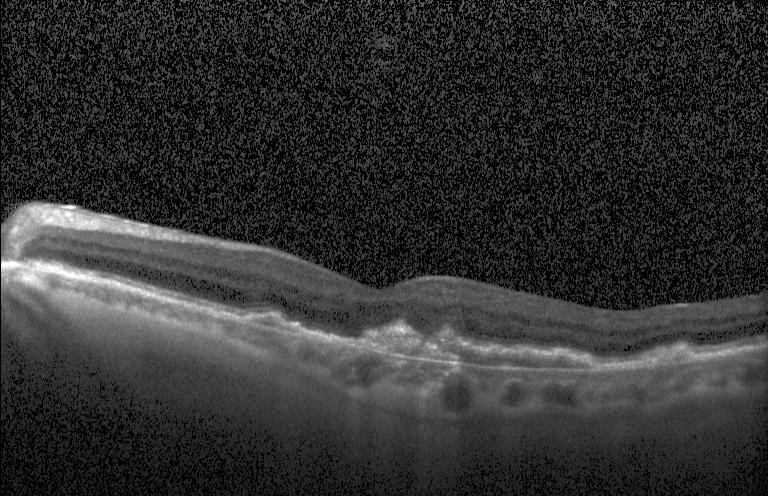
Heidelberg Spectralis OCT system · optical coherence tomography scan — OCT finding: a choroidal neovascular membrane.